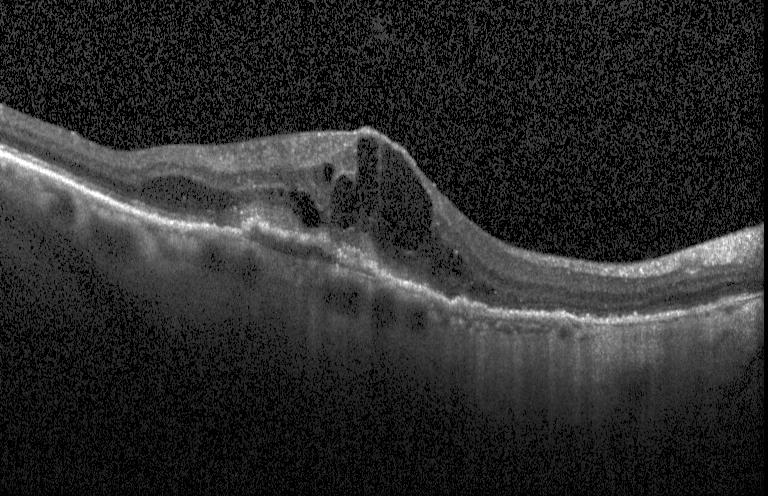 Retinal OCT B-scan.
This B-scan demonstrates CNV.